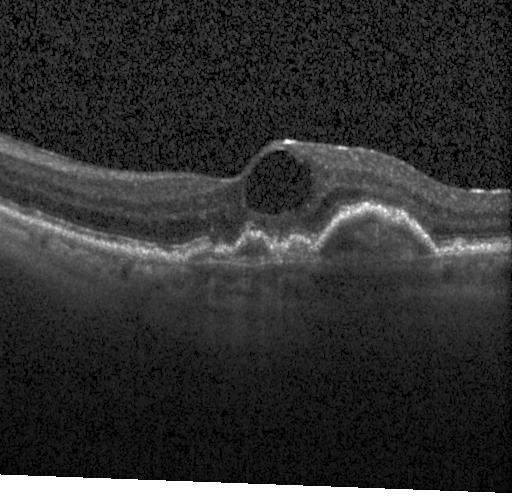
OCT scan showing a choroidal neovascular membrane.